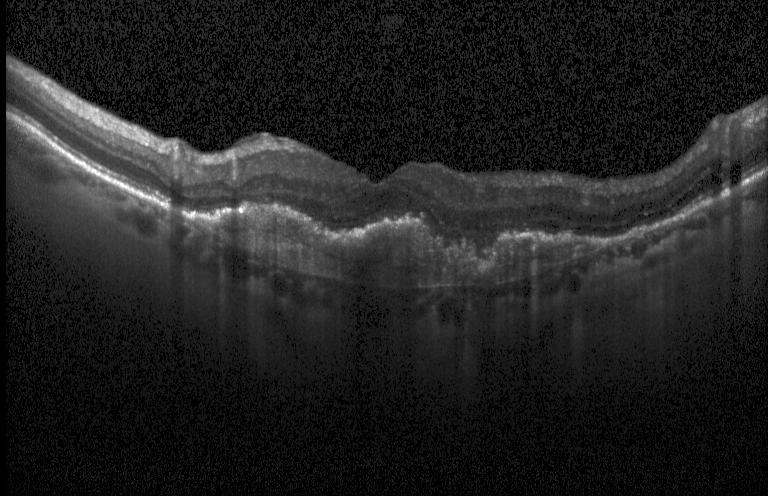 Diagnosis: a choroidal neovascular membrane.